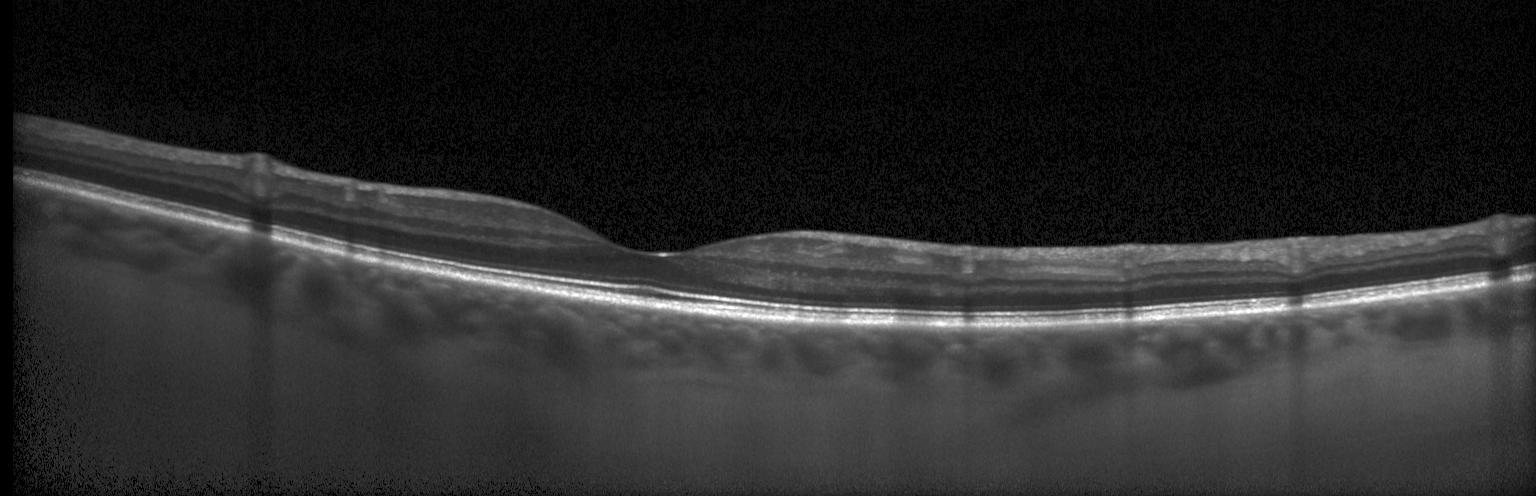

Centered on the fovea; spectral-domain optical coherence tomography; Heidelberg Spectralis; retinal OCT B-scan
Finding: no CNV, DME, or drusen.